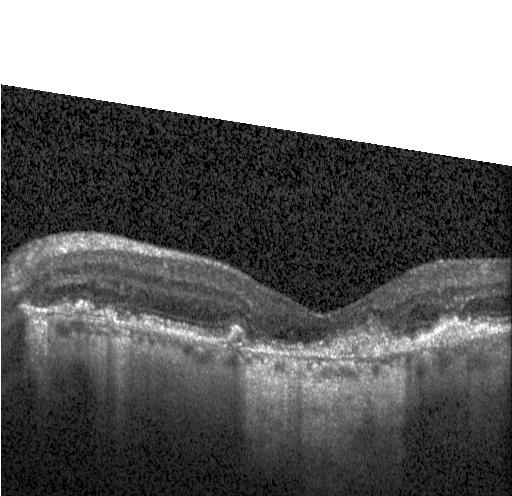

This B-scan demonstrates a choroidal neovascular membrane.